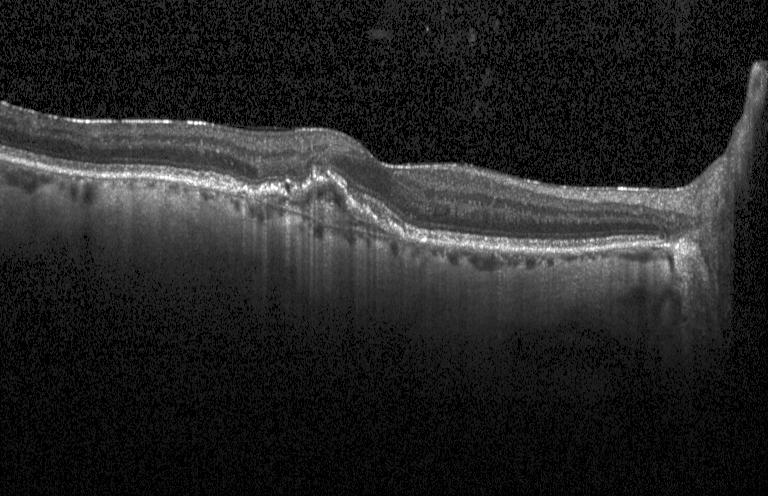

This B-scan demonstrates a choroidal neovascular membrane.